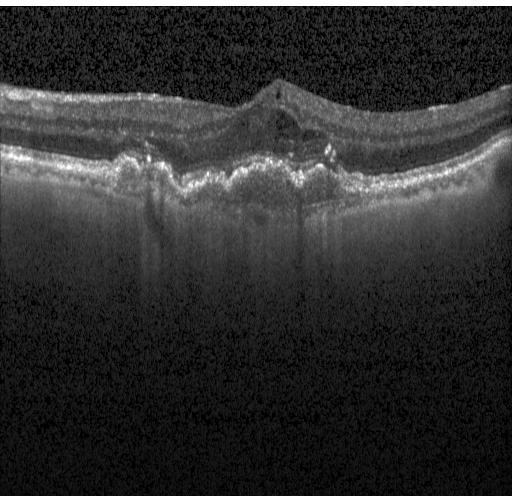

Diagnosis: choroidal neovascularization (CNV).